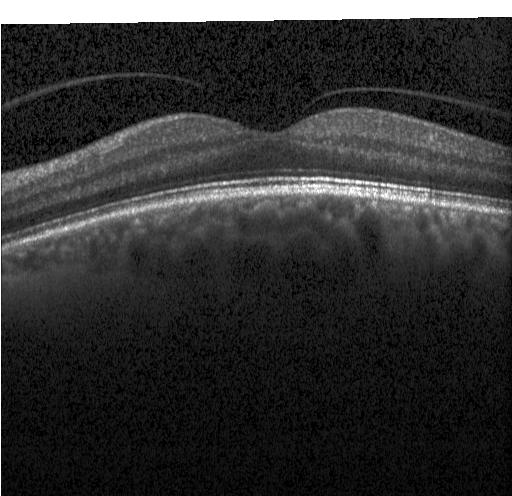
SD-OCT. Optical coherence tomography B-scan
This B-scan demonstrates neither choroidal neovascularization, diabetic macular edema, nor drusen.